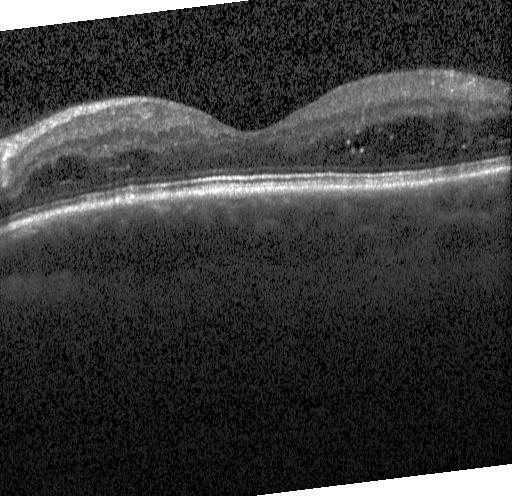
Instrument: Heidelberg Spectralis · optical coherence tomography B-scan · horizontal scan through the fovea
Finding: DME.